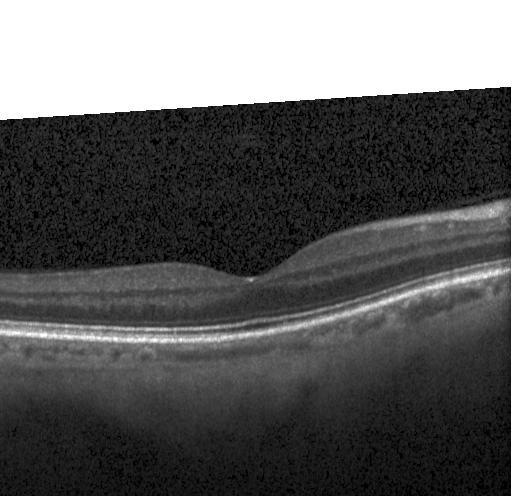 OCT finding: neither choroidal neovascularization, diabetic macular edema, nor drusen.